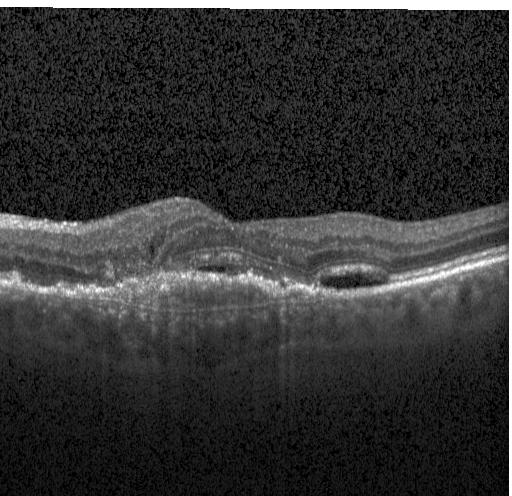

Macular scan; optical coherence tomography scan.
Finding: choroidal neovascularization.